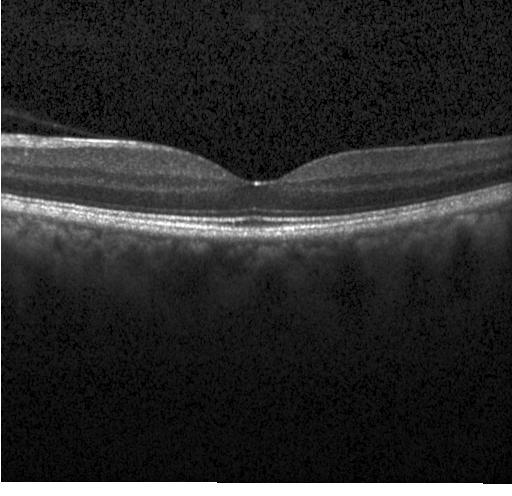
Spectral-domain optical coherence tomography, instrument: Heidelberg Spectralis, retinal OCT cross-section.
Finding: no evidence of CNV, DME, or drusen.